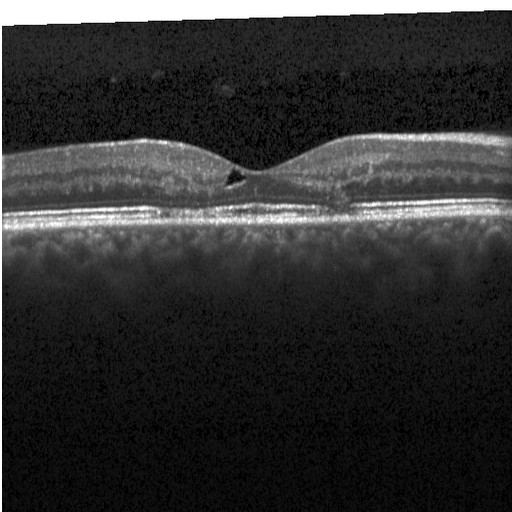 OCT B-scan showing diabetic macular edema.